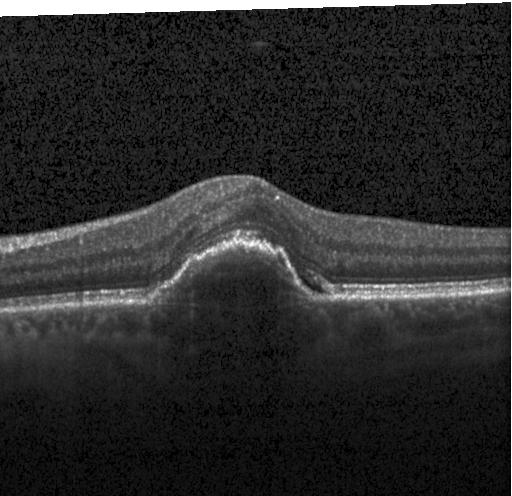 OCT line scan · macular scan · spectral-domain OCT.
The scan shows a choroidal neovascular membrane.